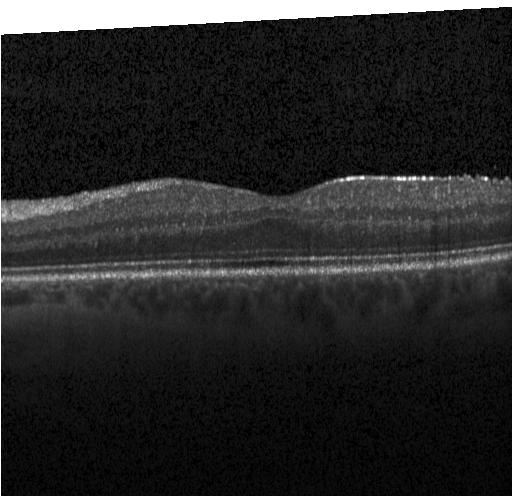

OCT B-scan.
Finding: no CNV, DME, or drusen.